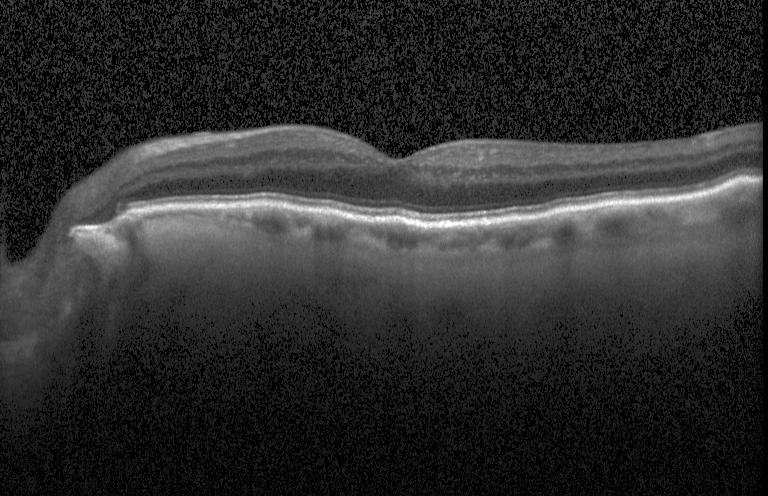
Macular OCT: no evidence of choroidal neovascularization, diabetic macular edema, or drusen.